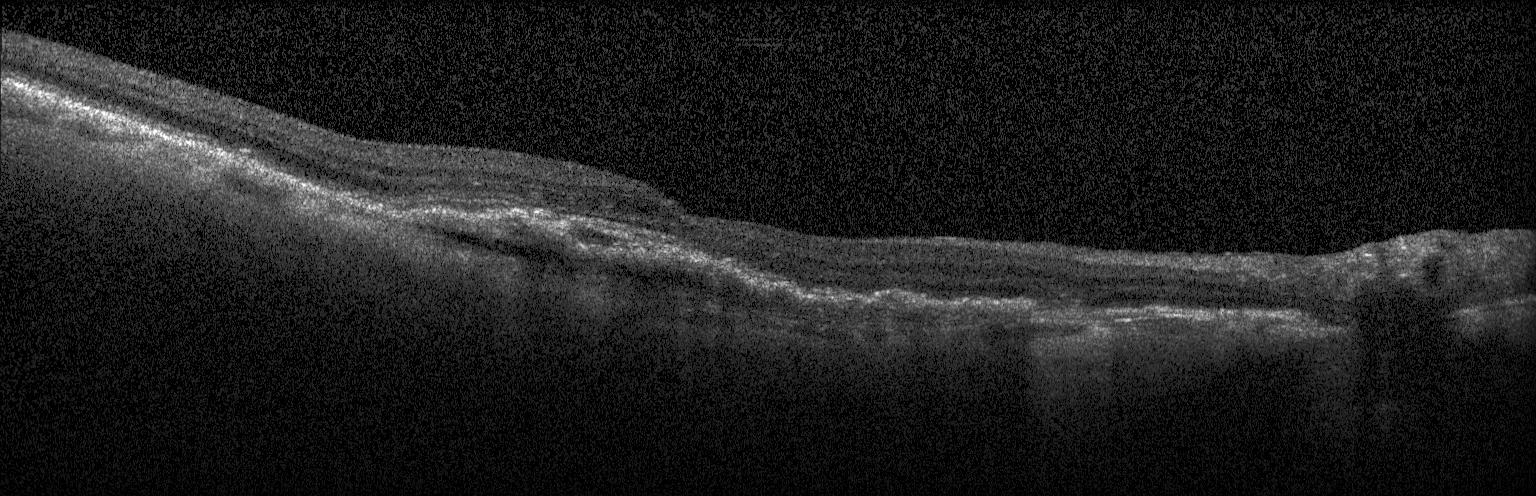
Diagnosis: choroidal neovascularization.